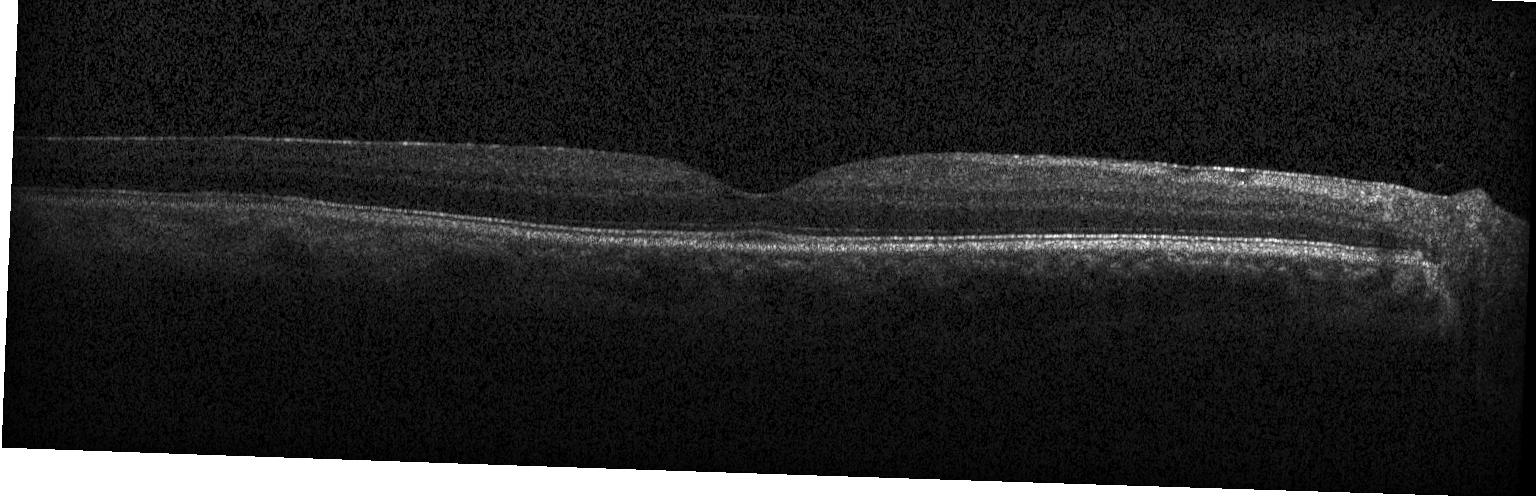 Finding: no choroidal neovascularization, no diabetic macular edema, and no drusen.